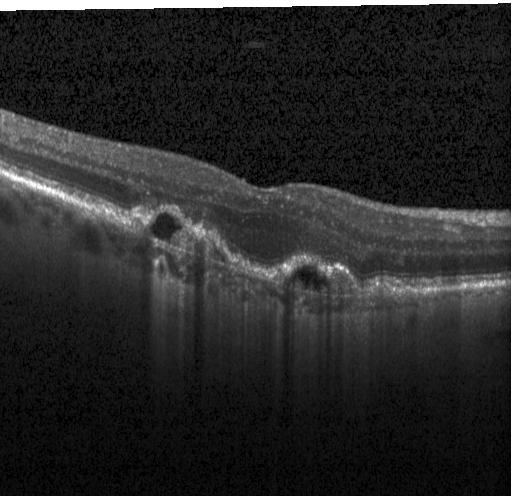 Horizontal scan through the fovea · retinal OCT cross-section · SD-OCT.
A choroidal neovascular membrane.